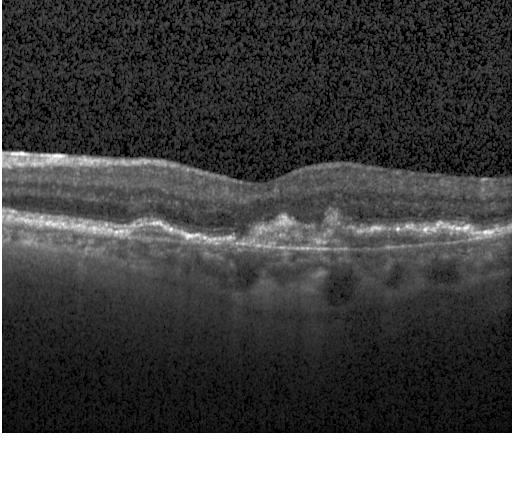 Spectral-domain optical coherence tomography, optical coherence tomography scan, instrument: Heidelberg Spectralis. A choroidal neovascular membrane.